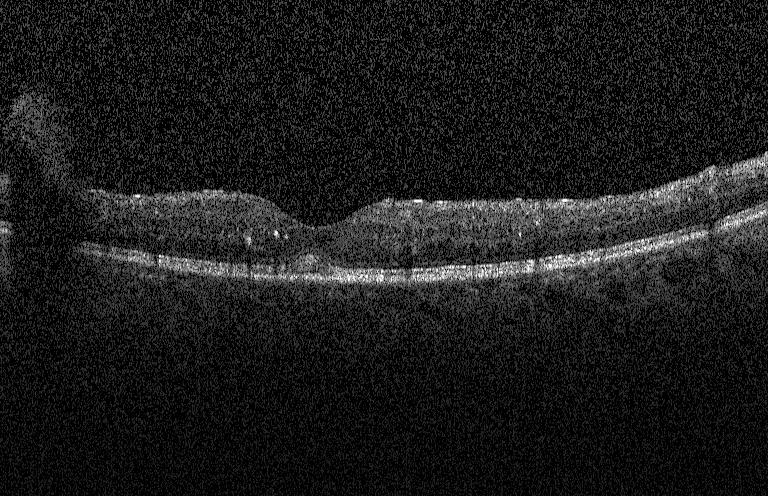

Retinal OCT cross-section — No CNV, DME, or drusen.